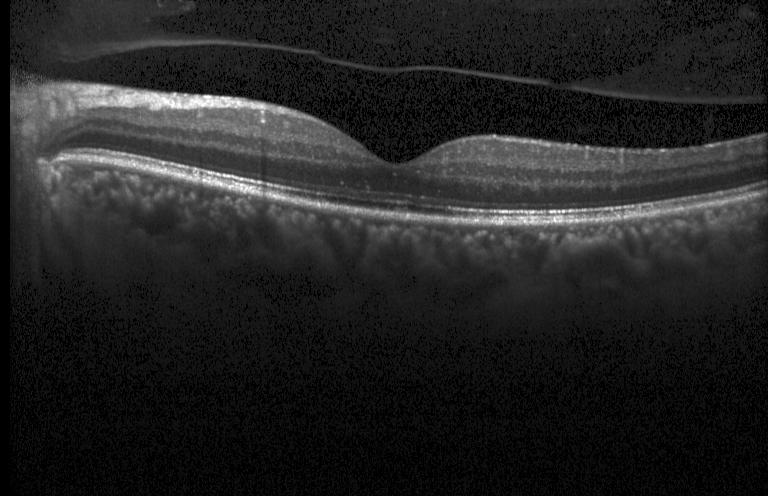

Heidelberg Spectralis OCT system. Retinal OCT cross-section
Assessment: no CNV, no DME, and no drusen.